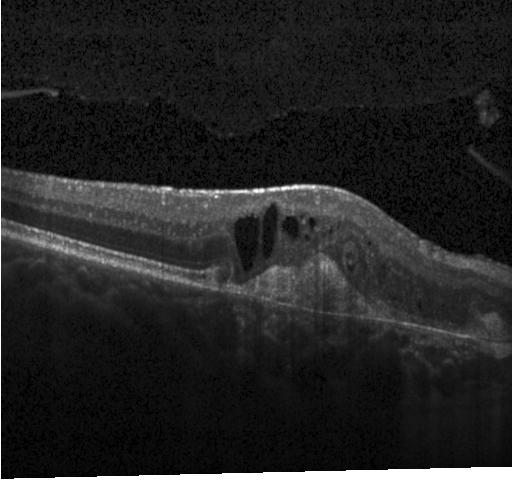
Through the macula, optical coherence tomography scan.
Finding: choroidal neovascularization (CNV).